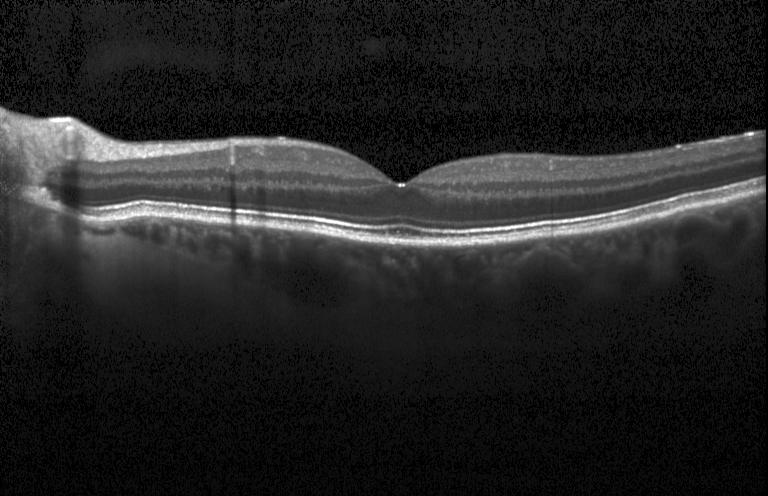
Optical coherence tomography B-scan.
The scan shows neither choroidal neovascularization, diabetic macular edema, nor drusen.